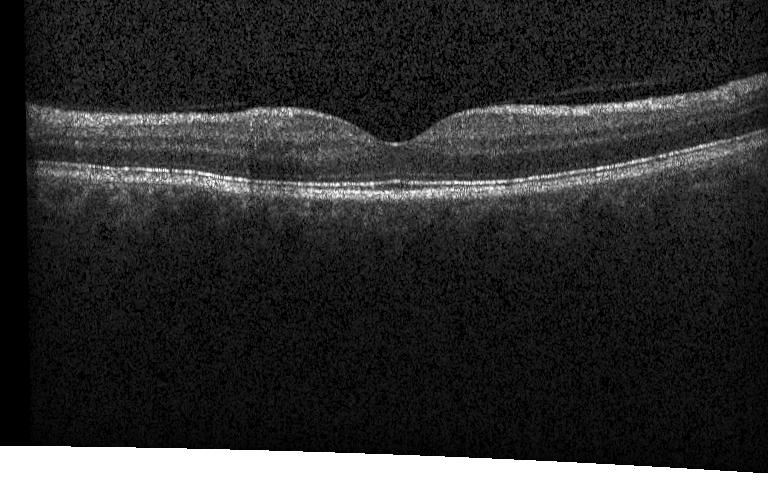 OCT line scan. Spectral-domain OCT. Centered on the fovea.
Macular OCT: neither choroidal neovascularization, diabetic macular edema, nor drusen.